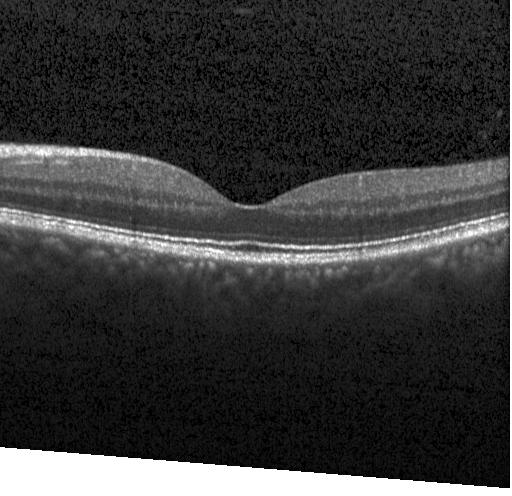
Retinal OCT cross-section · centered on the fovea
Impression: no evidence of CNV, DME, or drusen.